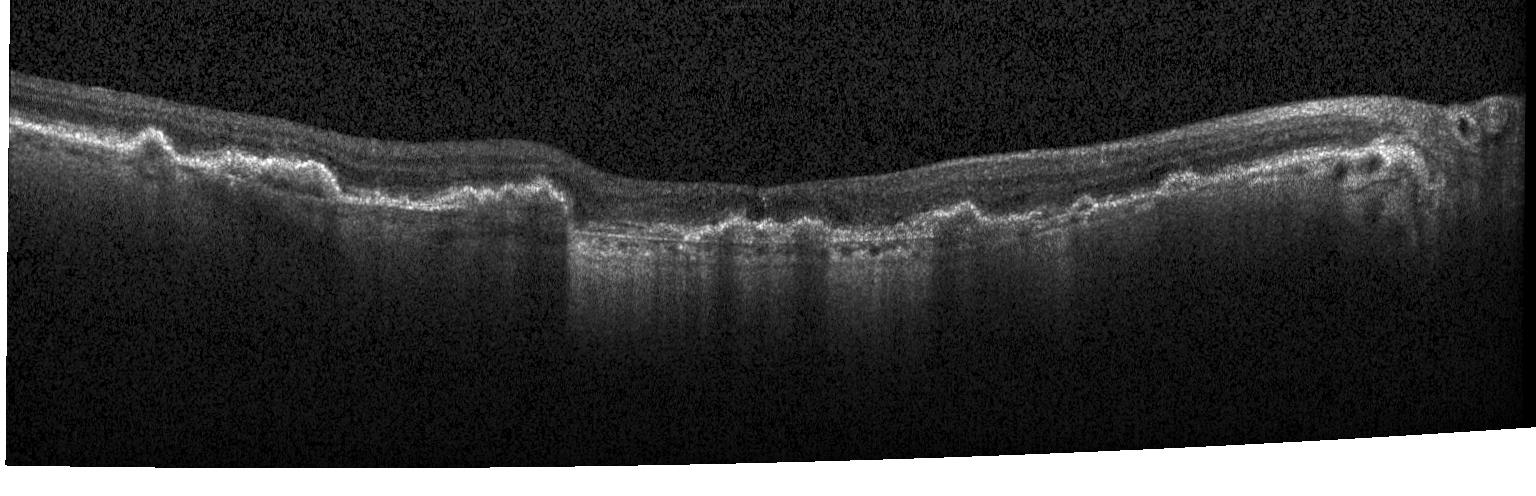 SD-OCT. Optical coherence tomography scan. Impression: choroidal neovascularization.